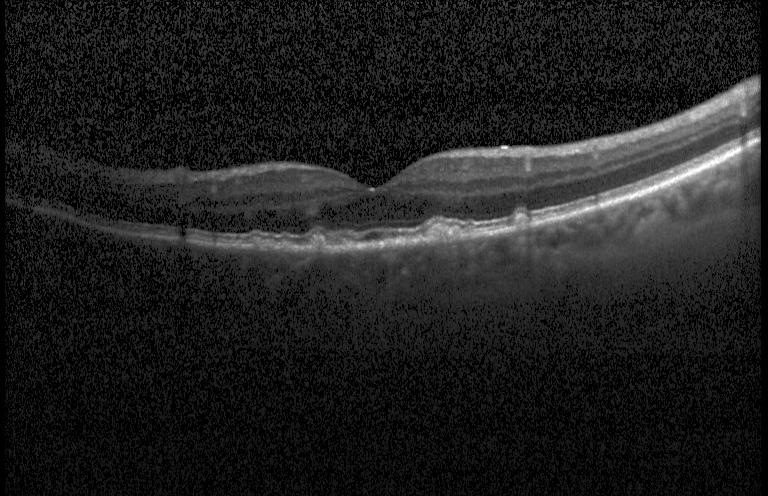
Spectral-domain OCT, retinal OCT cross-section. Diagnosis: drusen.